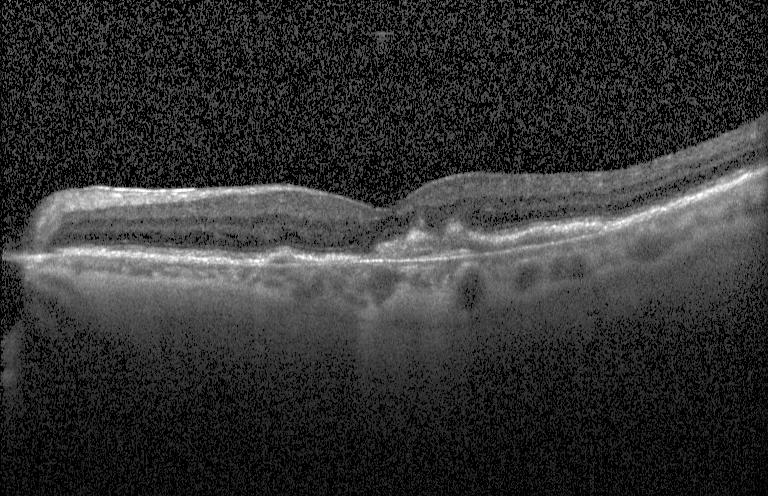 Optical coherence tomography B-scan, spectral-domain OCT — Assessment: CNV.